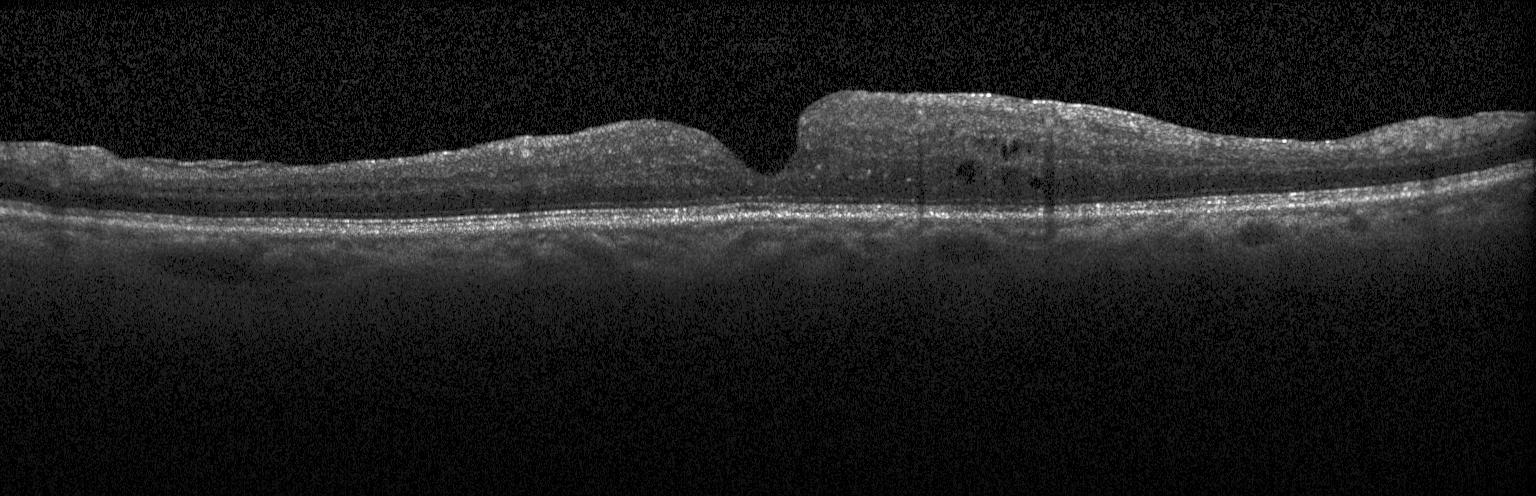
Spectral-domain optical coherence tomography · retinal OCT cross-section · horizontal scan through the fovea · Heidelberg Spectralis OCT system. Diabetic macular edema (DME).